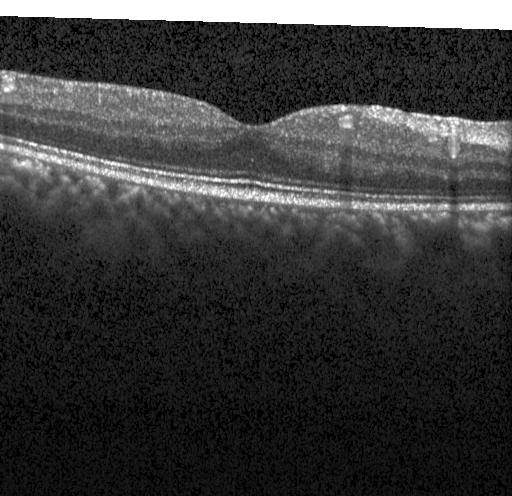
Through the macula. Optical coherence tomography scan. Dx: no evidence of CNV, DME, or drusen.